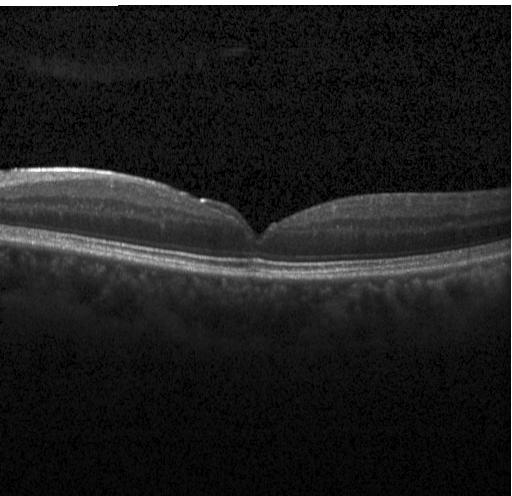
No CNV, no DME, and no drusen.